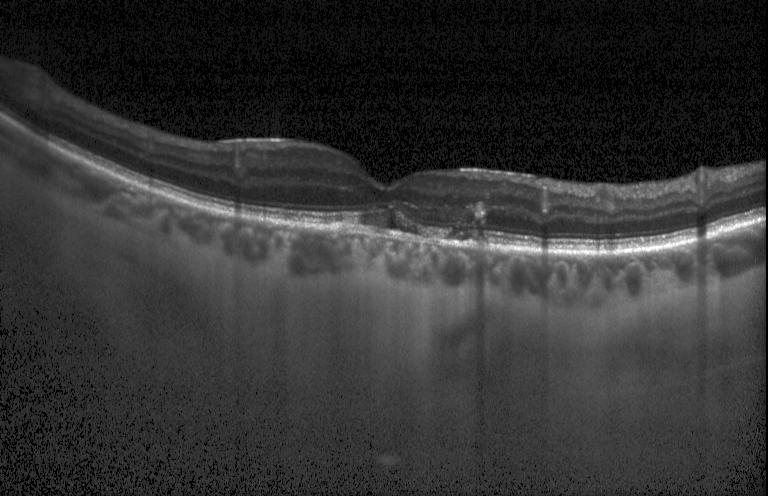

Through the macula; SD-OCT; instrument: Heidelberg Spectralis; OCT B-scan.
Finding: CNV.